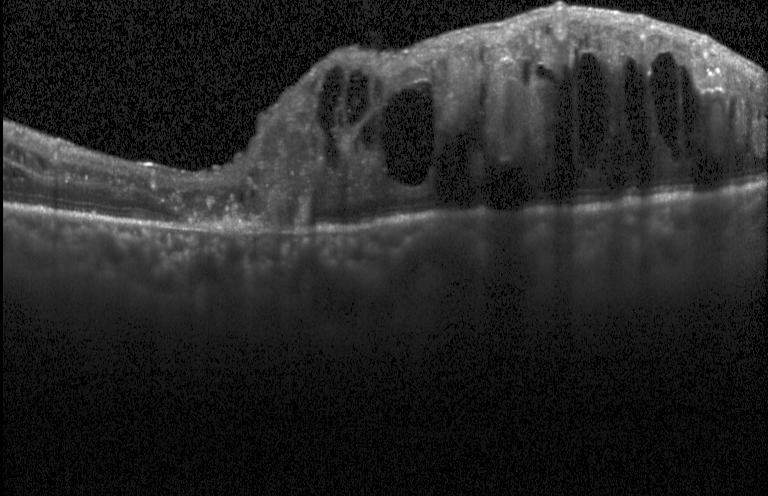 Optical coherence tomography B-scan.
Diagnosis: diabetic macular edema (DME).